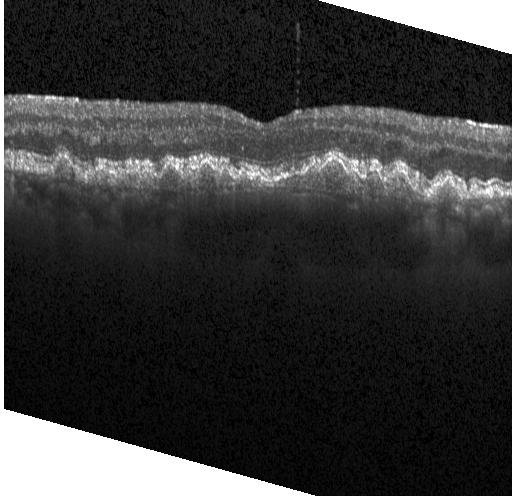

Retinal OCT cross-section, spectral-domain optical coherence tomography, macular scan, Heidelberg Spectralis OCT system — Diagnosis: choroidal neovascularization (CNV).